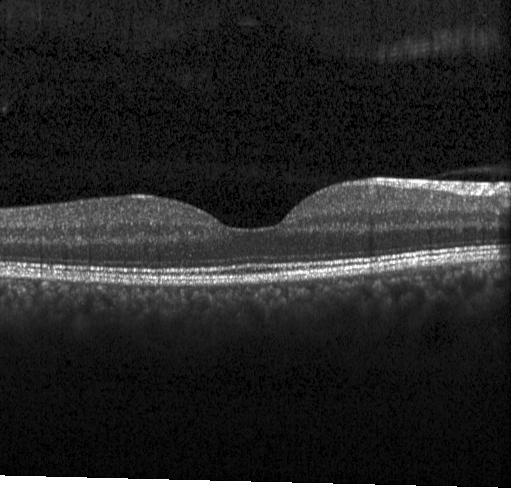

Optical coherence tomography scan.
Finding: no evidence of choroidal neovascularization, diabetic macular edema, or drusen.